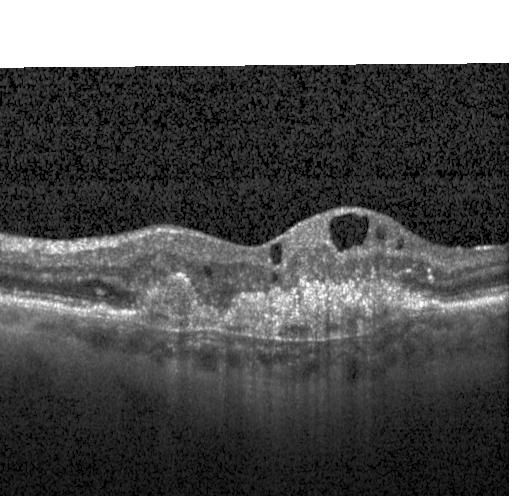
Impression: choroidal neovascularization (CNV).